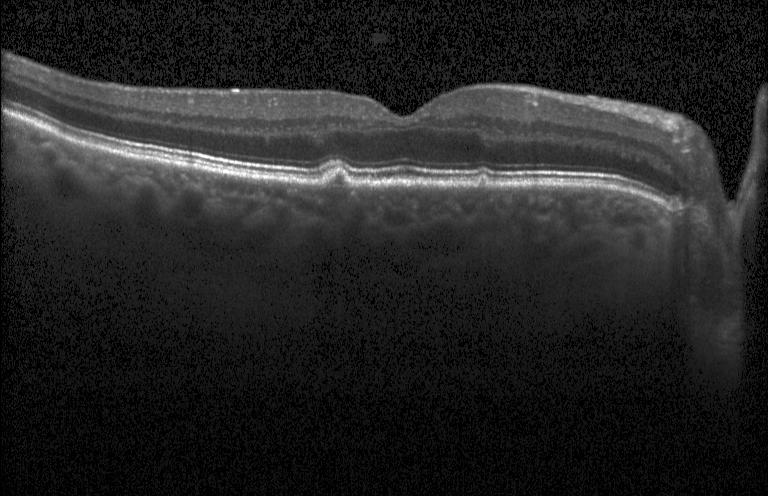
Macular OCT: sub-RPE drusenoid deposits.